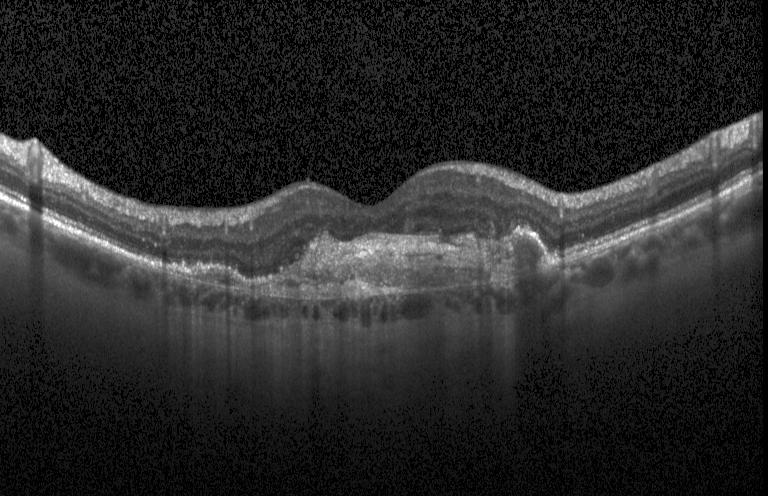 OCT B-scan
A choroidal neovascular membrane.